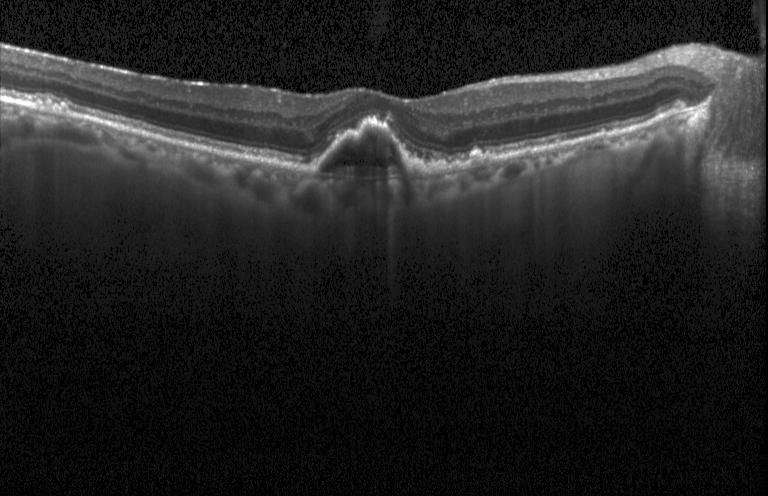
OCT B-scan showing a choroidal neovascular membrane.